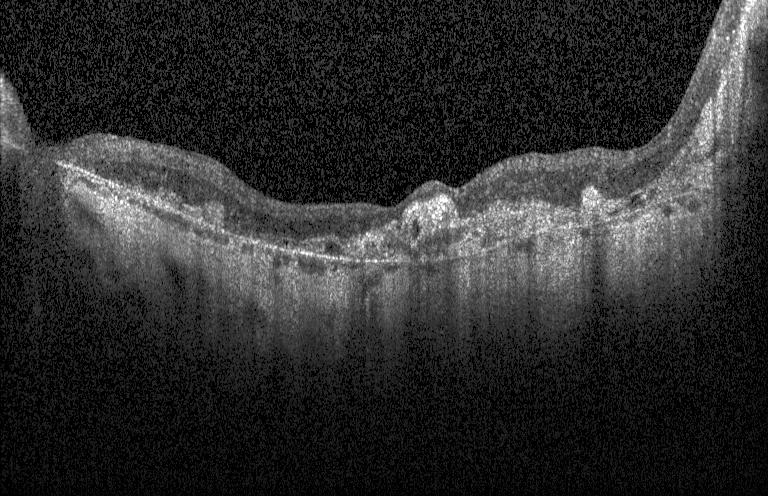

Retinal OCT B-scan. Heidelberg Spectralis. Spectral-domain OCT.
Diagnosis: choroidal neovascularization (CNV).